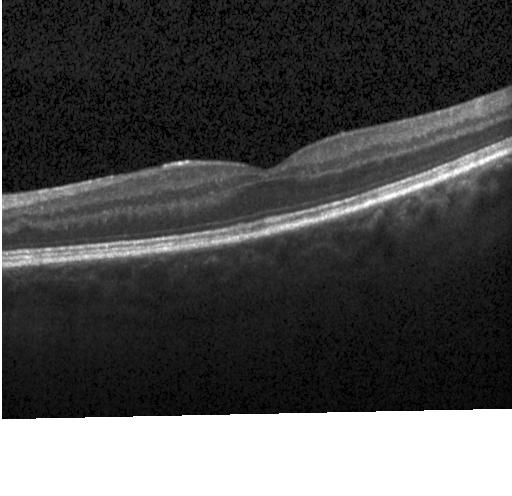
Centered on the fovea, Heidelberg Spectralis OCT system, retinal OCT B-scan.
The scan shows no CNV, DME, or drusen.